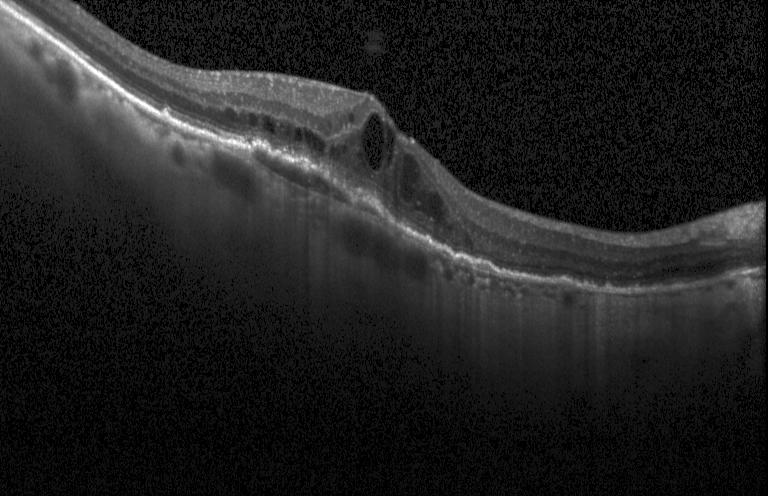

Finding: choroidal neovascularization (CNV).